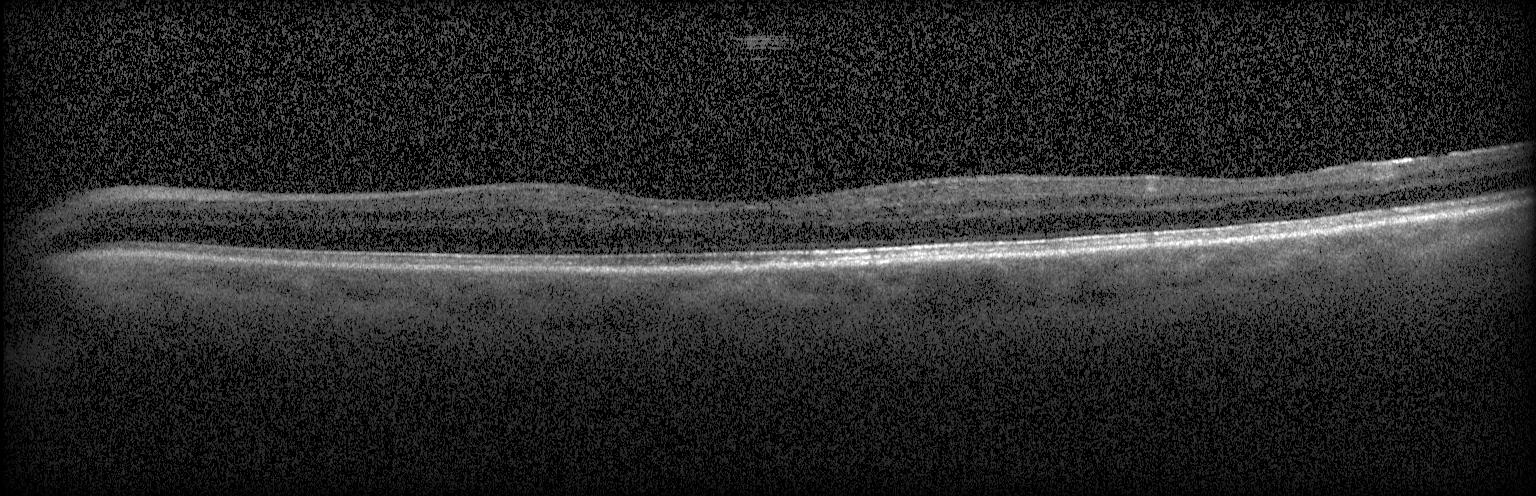 Optical coherence tomography B-scan; spectral-domain optical coherence tomography; Heidelberg Spectralis
This B-scan demonstrates neither CNV, DME, nor drusen.